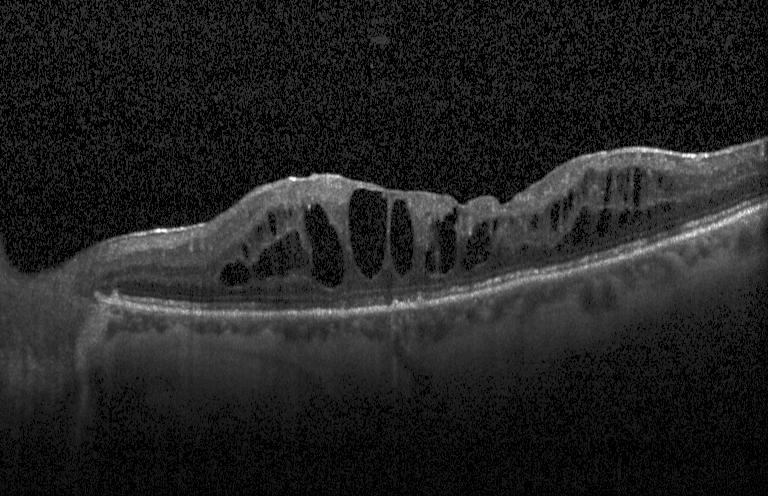 OCT B-scan
This B-scan demonstrates DME.